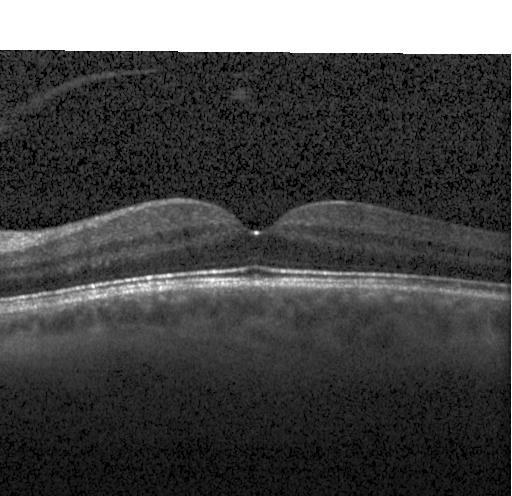
Impression: no CNV, no DME, and no drusen.